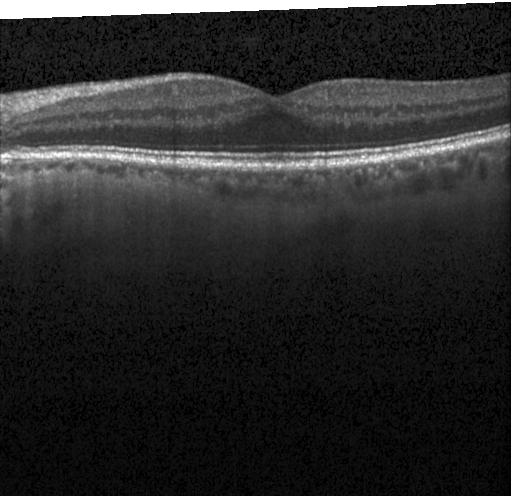
OCT B-scan — Neither choroidal neovascularization, diabetic macular edema, nor drusen.